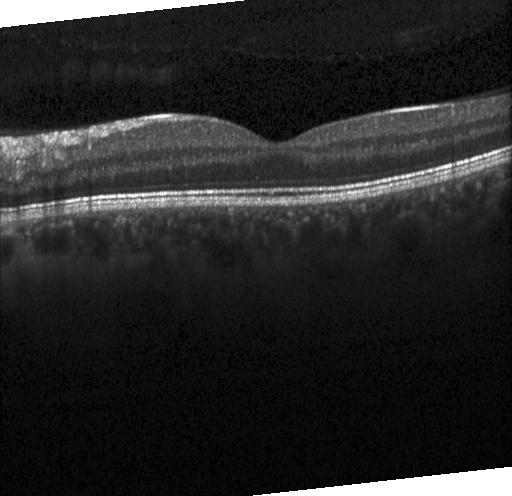

Diagnosis: no choroidal neovascularization, diabetic macular edema, or drusen.